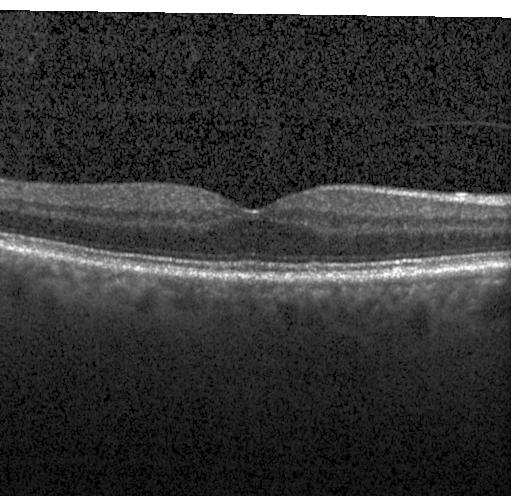

OCT B-scan.
Diagnosis: no evidence of CNV, DME, or drusen.